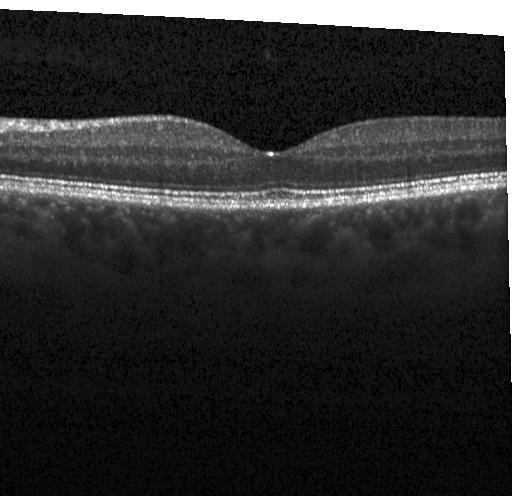 Instrument: Heidelberg Spectralis; SD-OCT; OCT line scan; fovea-centered
The scan shows no choroidal neovascularization, diabetic macular edema, or drusen.